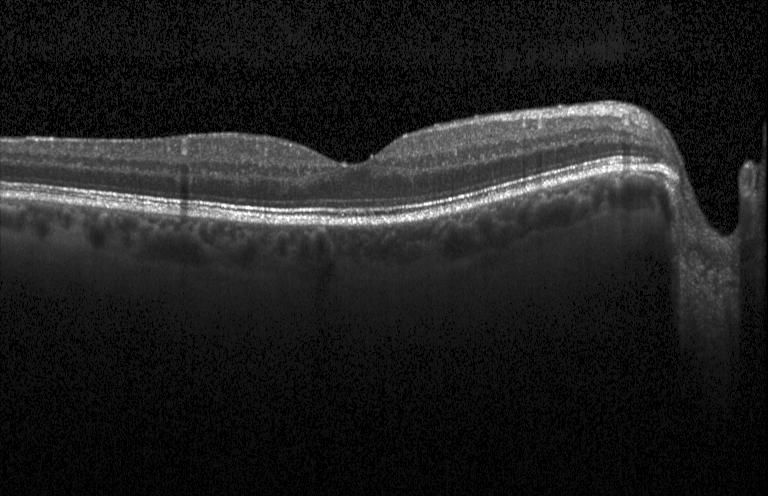
Spectral-domain optical coherence tomography. Macular scan. OCT B-scan.
Diagnosis: no evidence of choroidal neovascularization, diabetic macular edema, or drusen.